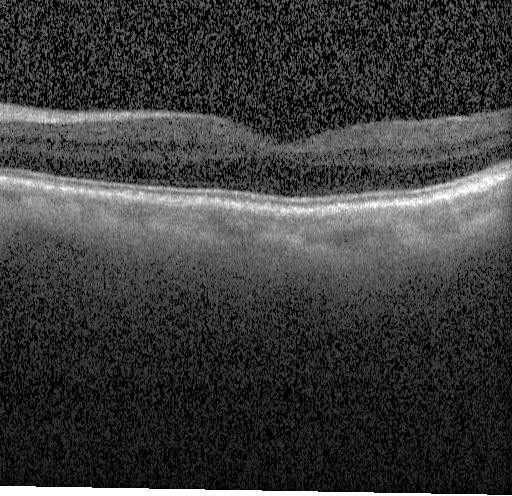 Optical coherence tomography B-scan.
Diagnosis: no choroidal neovascularization, diabetic macular edema, or drusen.